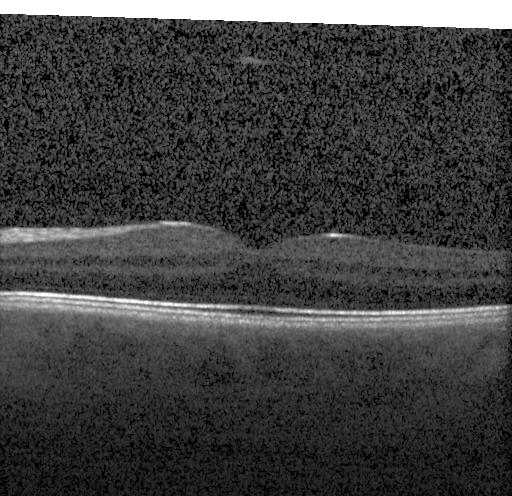

Heidelberg Spectralis OCT system, fovea-centered, optical coherence tomography scan, spectral-domain OCT.
Diagnosis: no choroidal neovascularization, no diabetic macular edema, and no drusen.